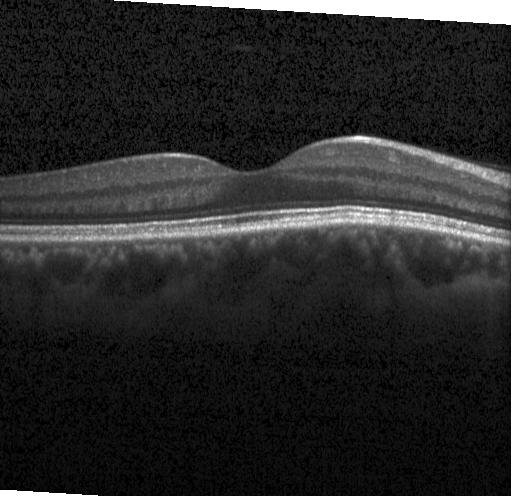

Macular OCT demonstrating no evidence of CNV, DME, or drusen.